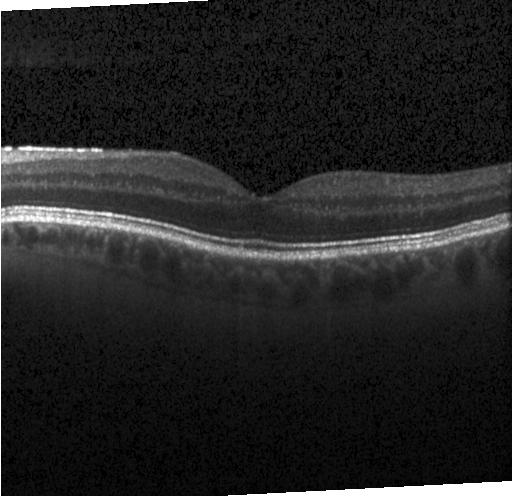
SD-OCT; retinal OCT cross-section
OCT finding: no choroidal neovascularization, no diabetic macular edema, and no drusen.